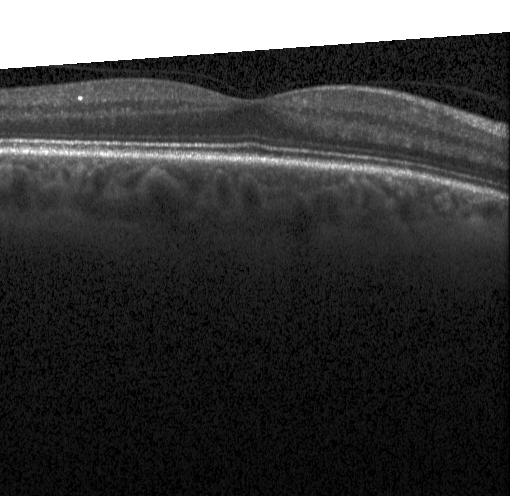
Optical coherence tomography B-scan — No evidence of CNV, DME, or drusen.